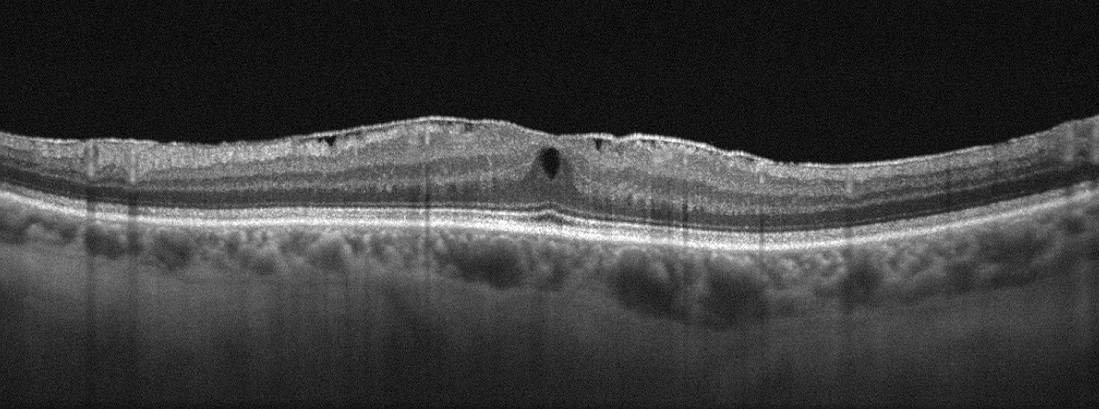

OCT B-scan · instrument: Optovue Avanti RTVue XR. Impression: epiretinal membrane.